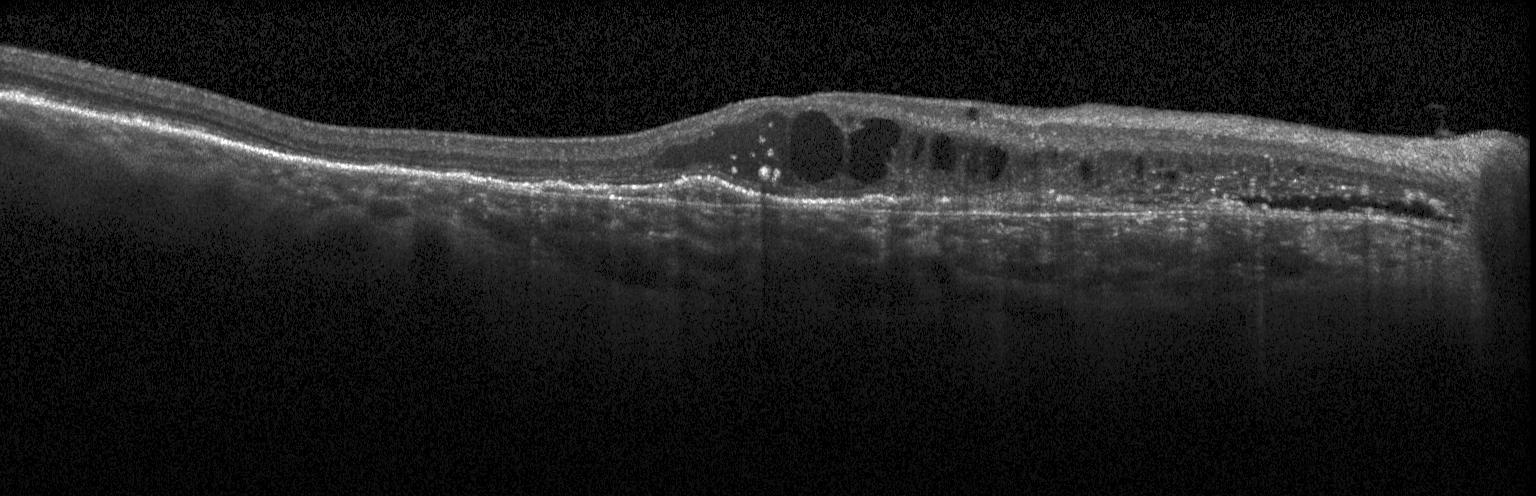

Macular OCT demonstrating a choroidal neovascular membrane.